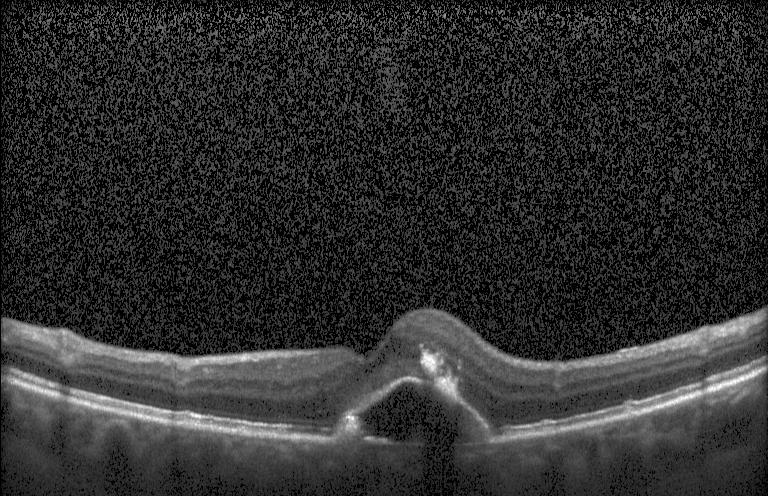
Spectral-domain OCT, retinal OCT B-scan
Diagnosis: choroidal neovascularization (CNV).